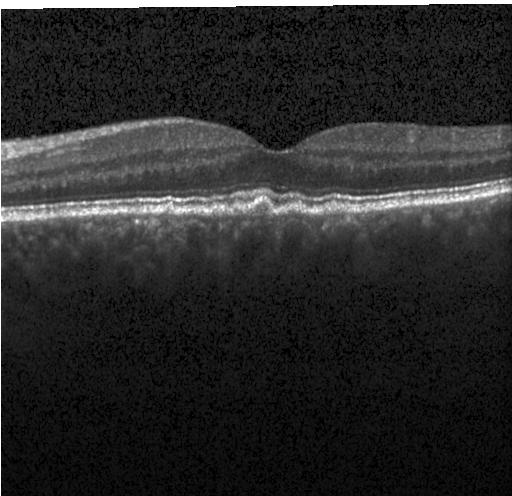
OCT line scan
Impression: sub-RPE drusenoid deposits.